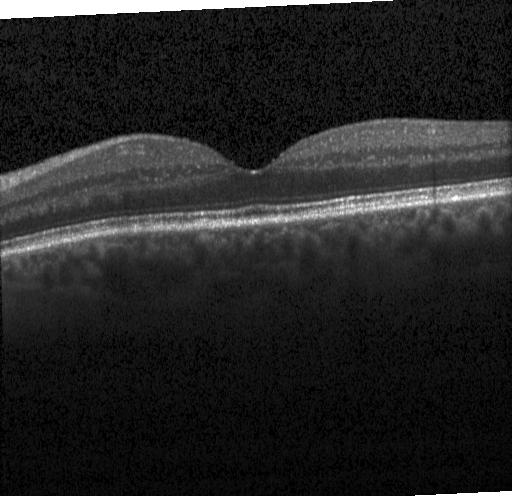
Spectral-domain OCT; Heidelberg Spectralis; horizontal scan through the fovea; OCT line scan.
No choroidal neovascularization, no diabetic macular edema, and no drusen.